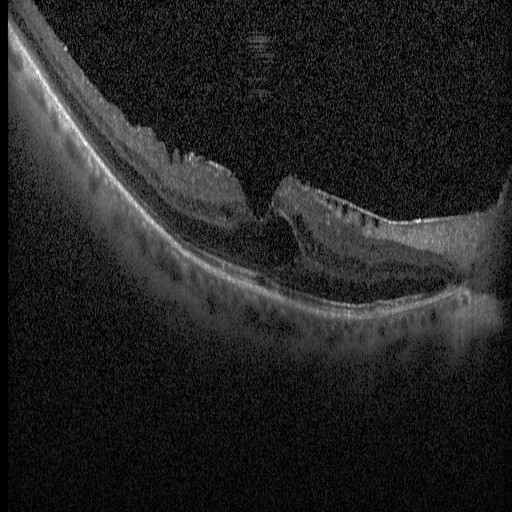
SD-OCT. OCT B-scan. Horizontal scan through the fovea. Acquired on a Heidelberg Spectralis — Macular OCT: diabetic macular edema.